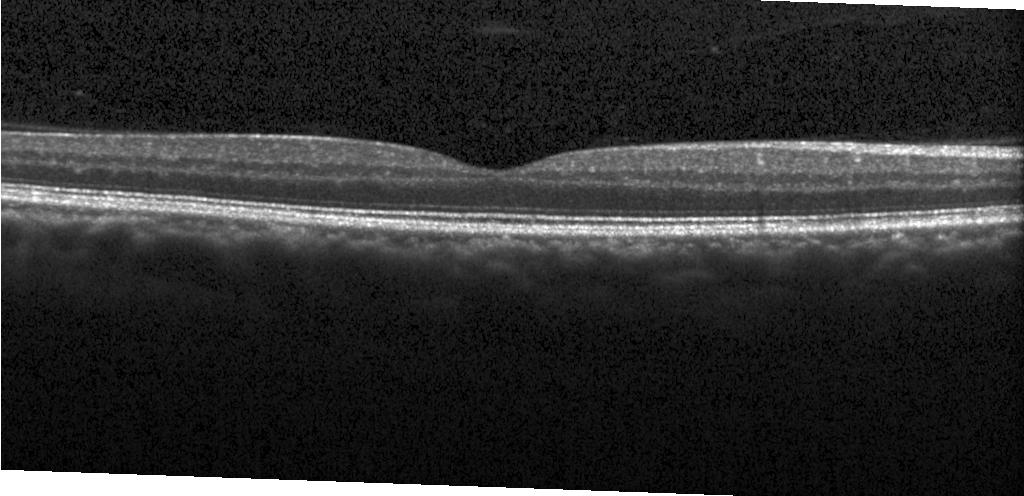

Optical coherence tomography scan; fovea-centered; spectral-domain optical coherence tomography; Heidelberg Spectralis.
Impression: neither choroidal neovascularization, diabetic macular edema, nor drusen.